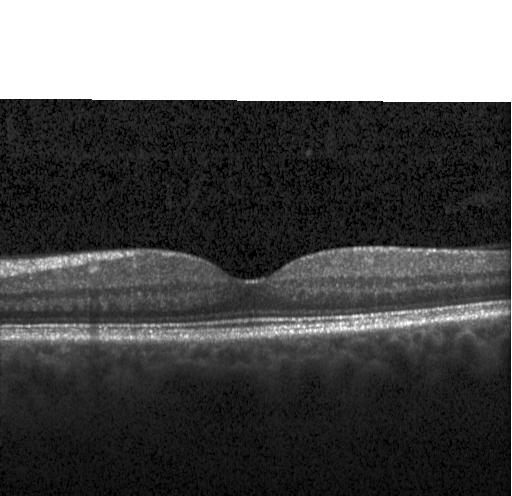
Optical coherence tomography scan. Horizontal scan through the fovea.
This B-scan demonstrates no evidence of choroidal neovascularization, diabetic macular edema, or drusen.